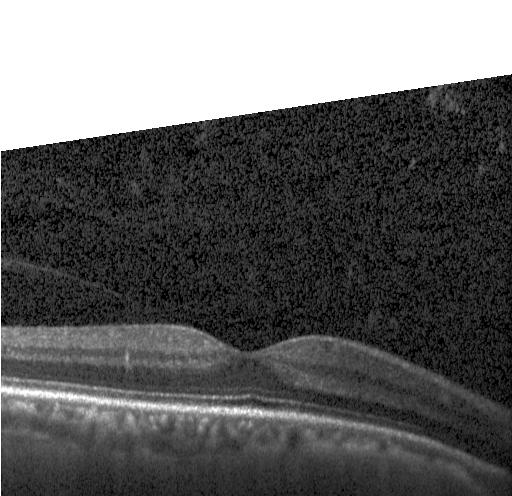

Retinal OCT B-scan.
Diagnosis: no choroidal neovascularization, diabetic macular edema, or drusen.